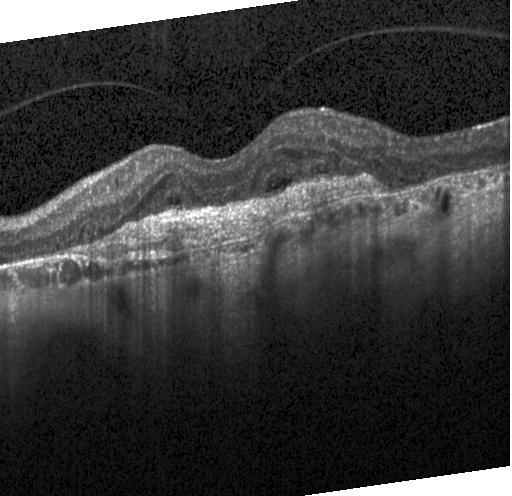 Finding: a choroidal neovascular membrane.